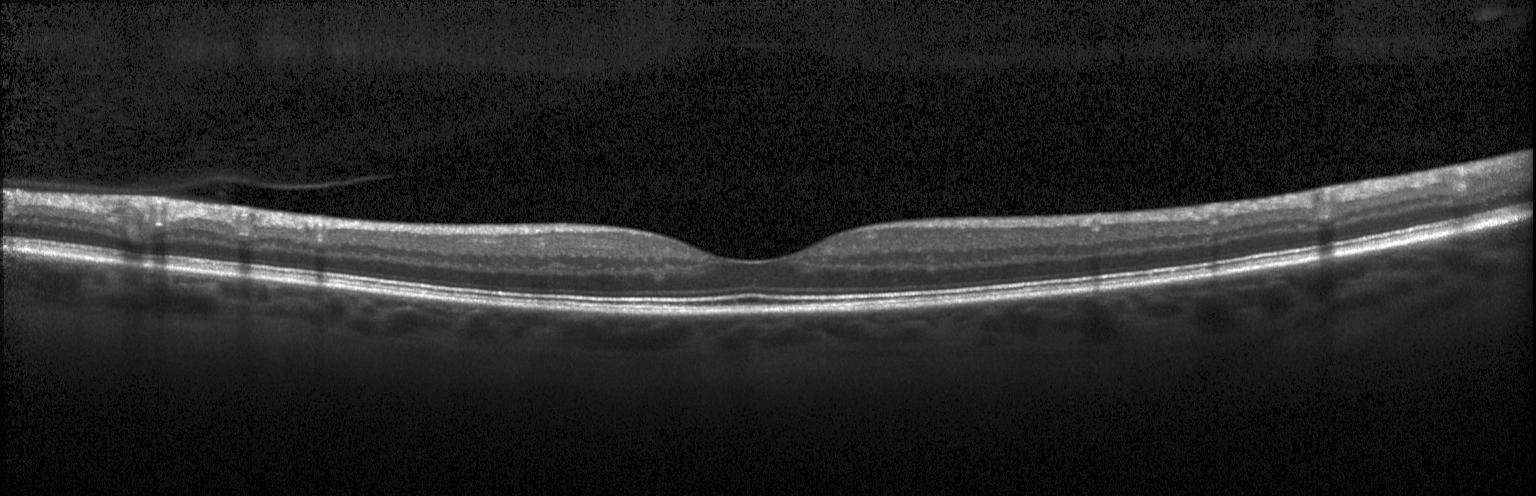
Diagnosis: no CNV, DME, or drusen.